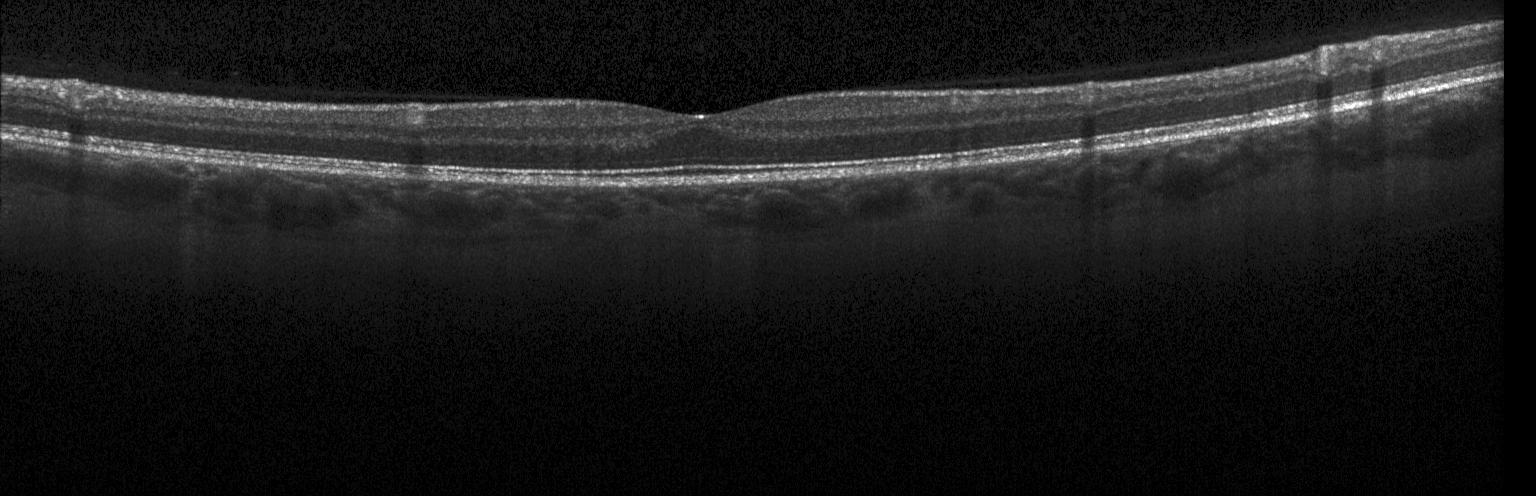 Spectral-domain optical coherence tomography, OCT B-scan, acquired on a Heidelberg Spectralis, macular scan
No choroidal neovascularization, no diabetic macular edema, and no drusen.